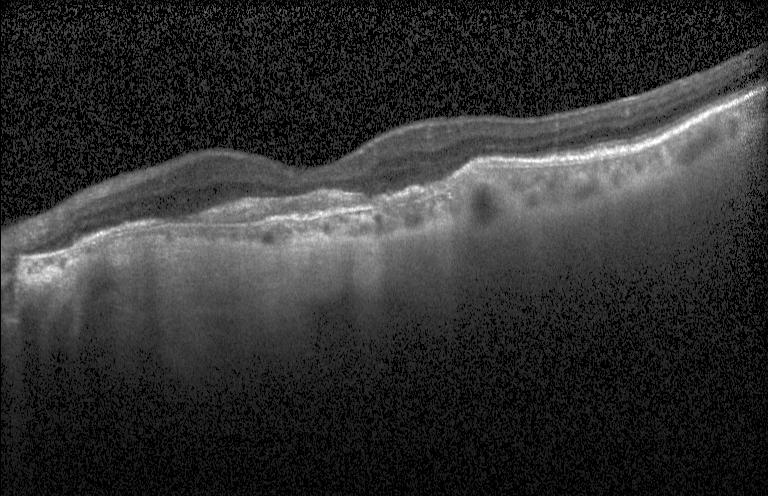
Optical coherence tomography B-scan — Finding: CNV.